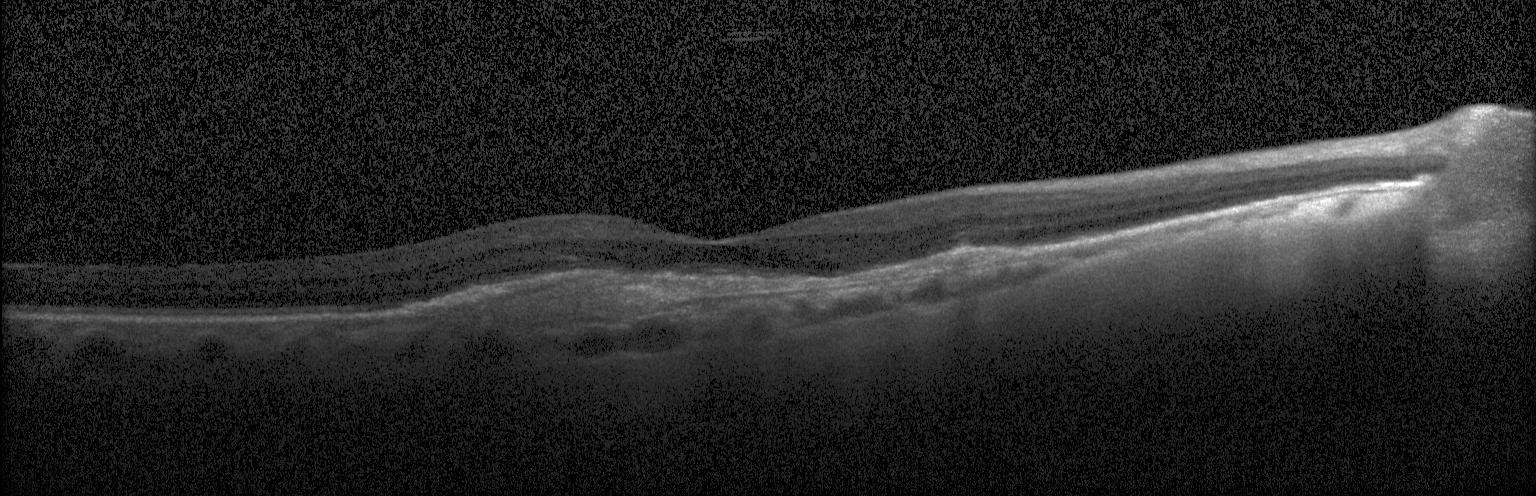

OCT line scan. Through the macula. Instrument: Heidelberg Spectralis
Diagnosis: CNV.